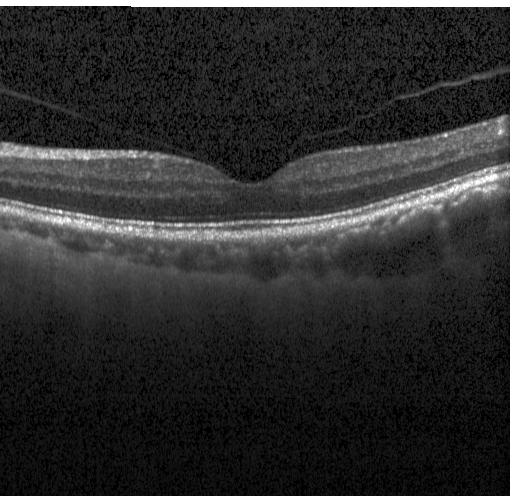 Instrument: Heidelberg Spectralis; macular scan; optical coherence tomography scan
Diagnosis: no choroidal neovascularization, no diabetic macular edema, and no drusen.